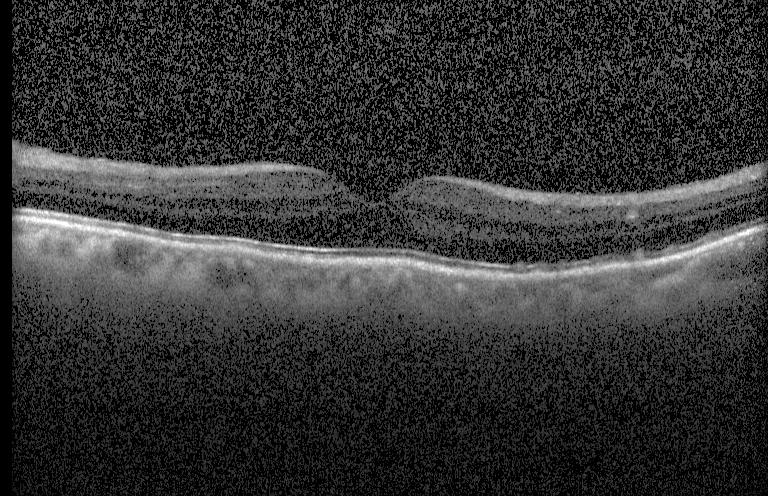
Optical coherence tomography scan — Impression: no choroidal neovascularization, diabetic macular edema, or drusen.